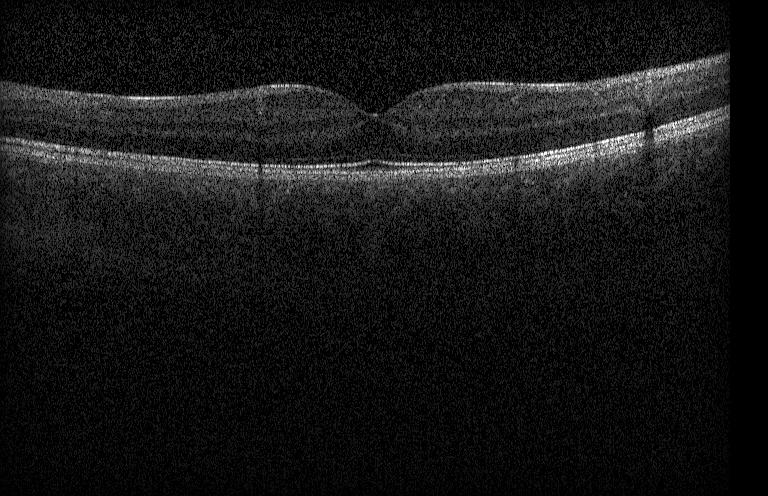
Acquired on a Heidelberg Spectralis; OCT line scan
Impression: no choroidal neovascularization, diabetic macular edema, or drusen.